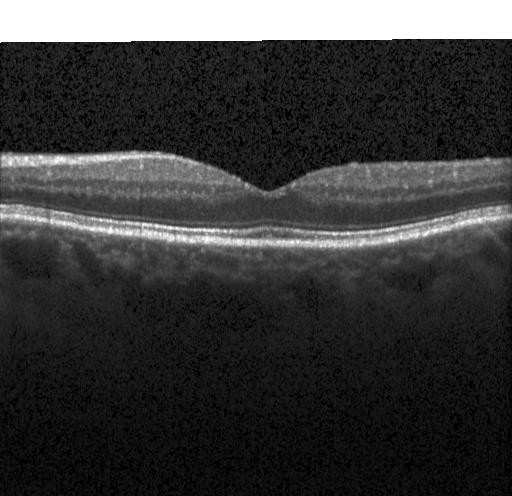

OCT B-scan; fovea-centered.
No choroidal neovascularization, no diabetic macular edema, and no drusen.